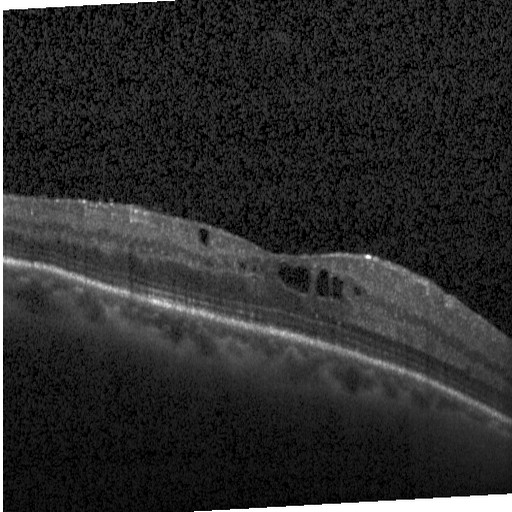 Impression: diabetic macular edema.